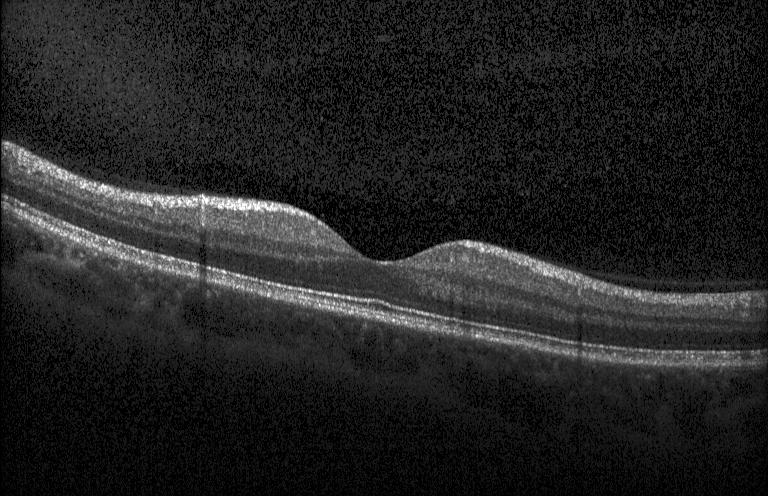

Fovea-centered; SD-OCT; Heidelberg Spectralis; optical coherence tomography scan — Finding: no evidence of choroidal neovascularization, diabetic macular edema, or drusen.